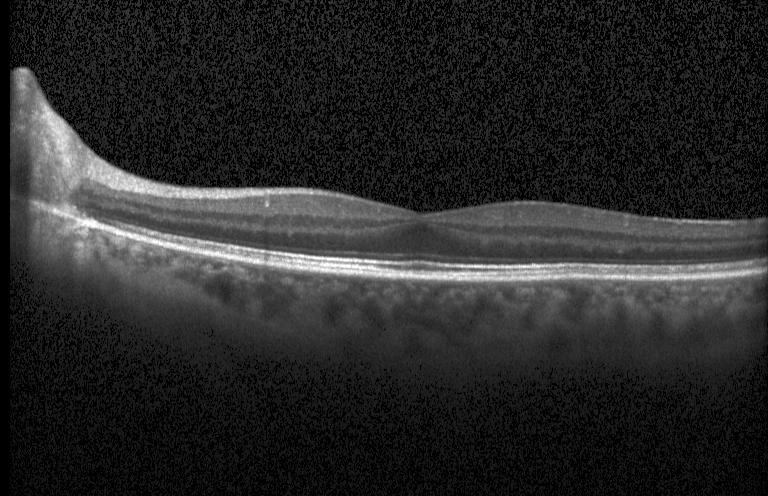 OCT scan showing neither CNV, DME, nor drusen.